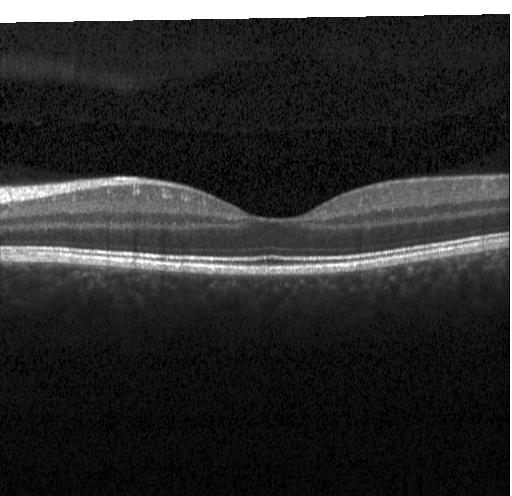 Optical coherence tomography B-scan — This B-scan demonstrates no CNV, DME, or drusen.